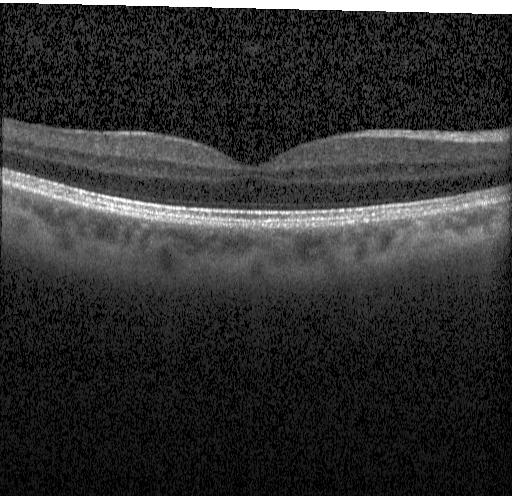

Finding: no choroidal neovascularization, diabetic macular edema, or drusen.